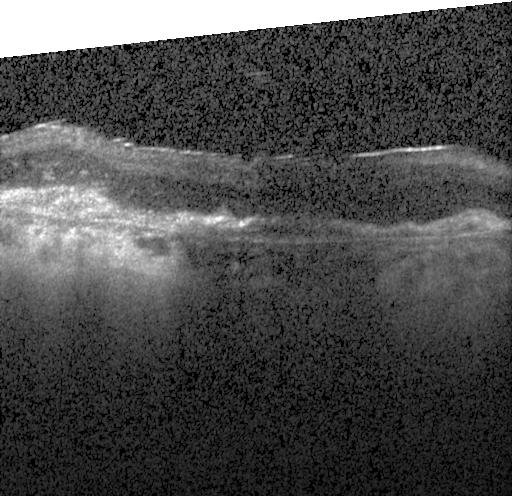 Macular scan. OCT line scan. Spectral-domain OCT. Acquired on a Heidelberg Spectralis.
The scan shows CNV.